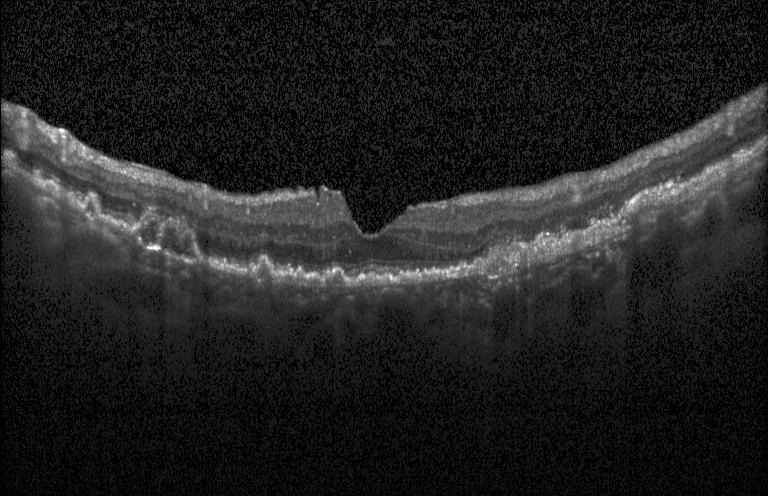 Acquired on a Heidelberg Spectralis. Retinal OCT cross-section. Spectral-domain optical coherence tomography. Horizontal scan through the fovea — Dx: CNV.